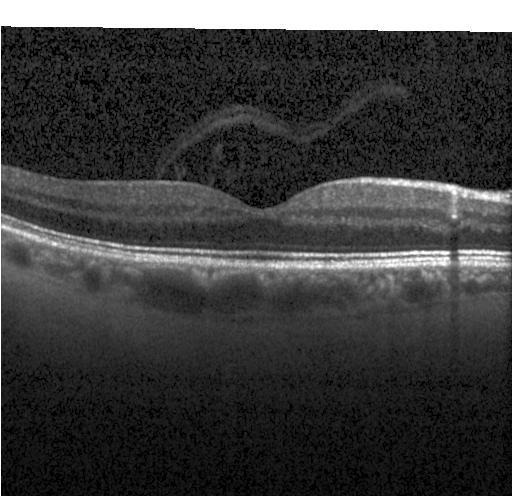
Heidelberg Spectralis. Optical coherence tomography scan. Horizontal scan through the fovea. Spectral-domain optical coherence tomography
Impression: no choroidal neovascularization, diabetic macular edema, or drusen.